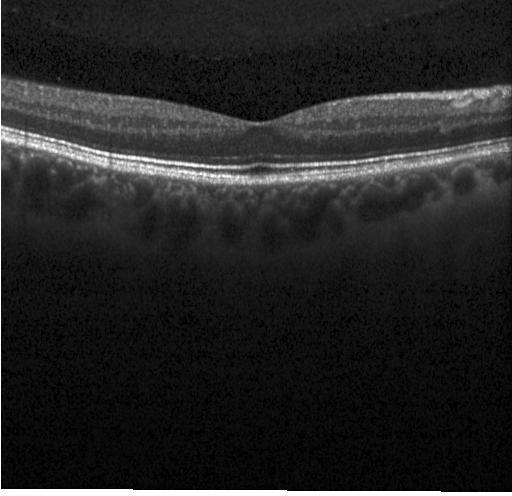
Diagnosis: no CNV, DME, or drusen.